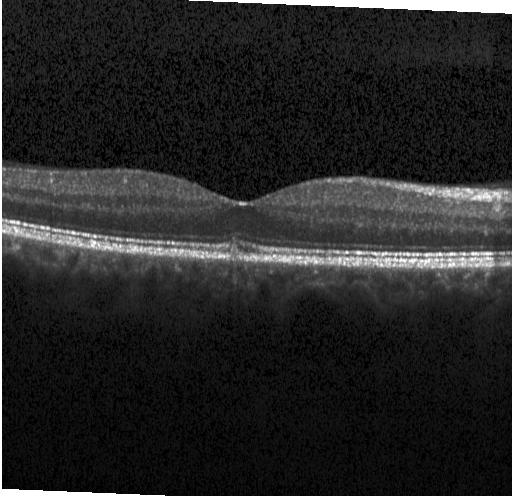 Optical coherence tomography scan — Impression: drusen.